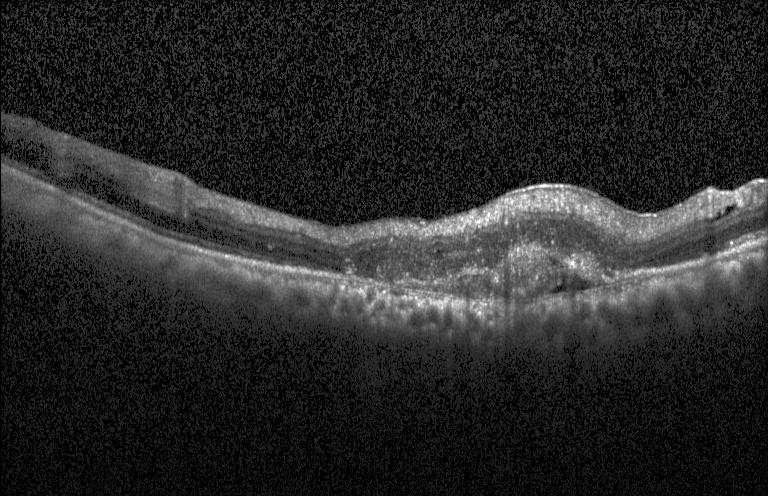 Diagnosis: a choroidal neovascular membrane.